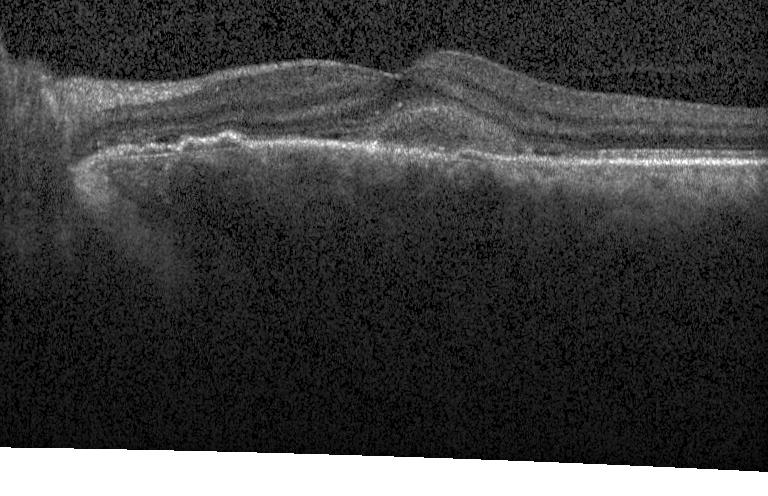

Retinal OCT B-scan · spectral-domain optical coherence tomography · macular scan. This B-scan demonstrates a choroidal neovascular membrane.